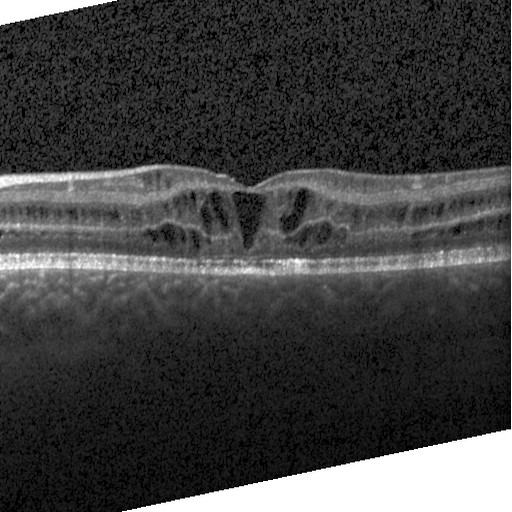

Heidelberg Spectralis; fovea-centered; OCT line scan; spectral-domain optical coherence tomography. Finding: diabetic macular edema.